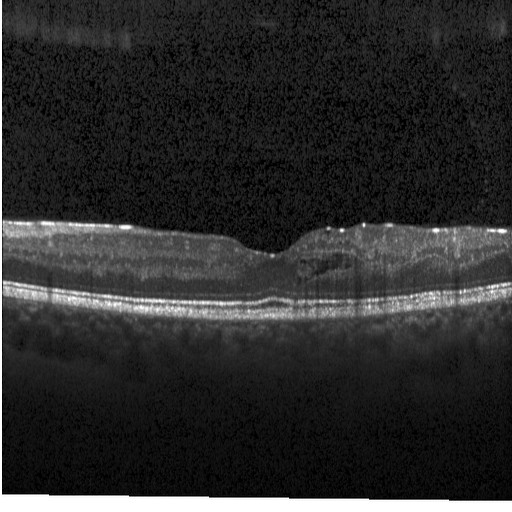
Fovea-centered. Optical coherence tomography scan. Acquired on a Heidelberg Spectralis. Assessment: diabetic macular edema (DME).